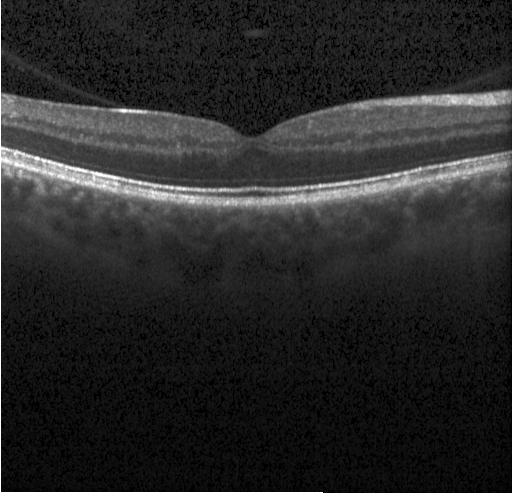

Impression: no choroidal neovascularization, diabetic macular edema, or drusen.